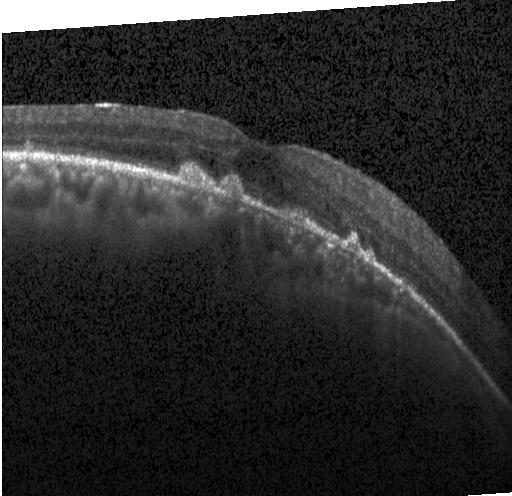 OCT B-scan.
Dx: drusen.